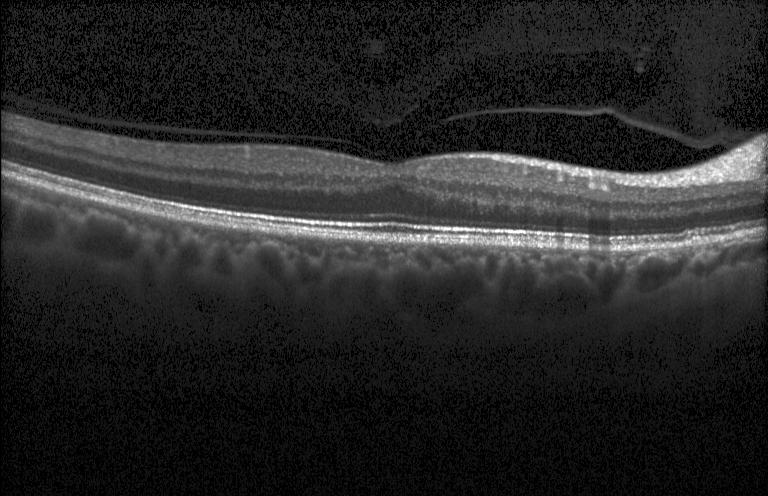

OCT scan showing no choroidal neovascularization, no diabetic macular edema, and no drusen.